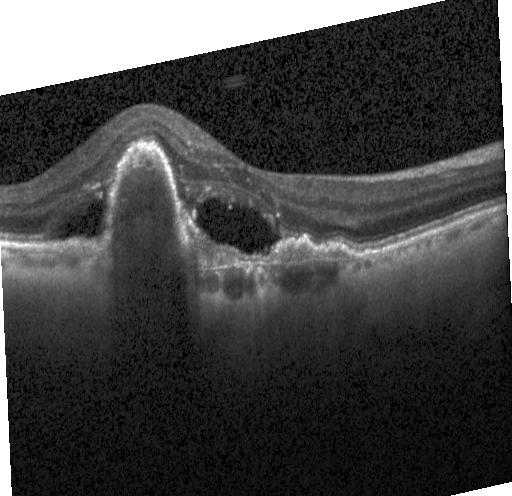

Finding: CNV.